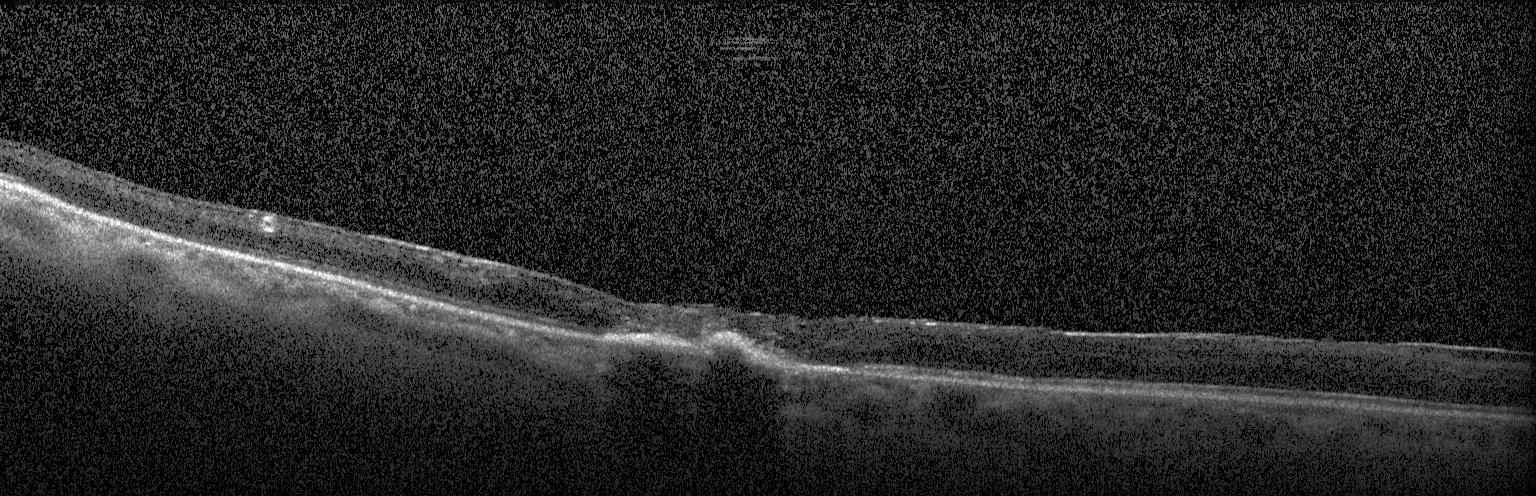
This B-scan demonstrates CNV.